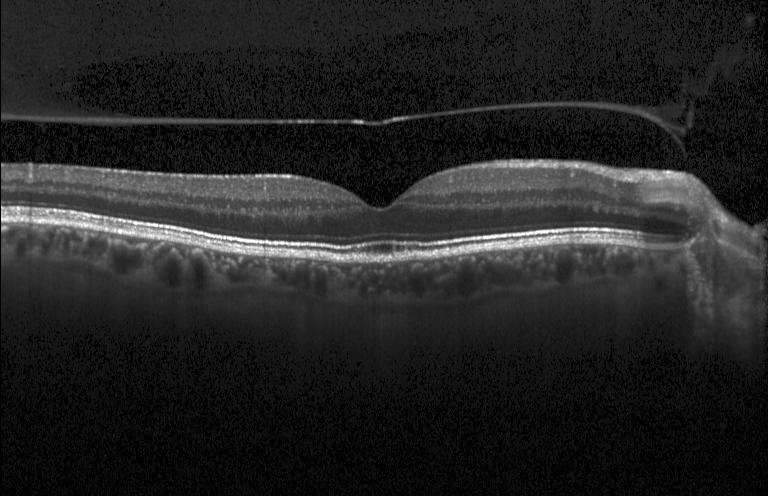
SD-OCT; macular scan; optical coherence tomography scan. Impression: no evidence of choroidal neovascularization, diabetic macular edema, or drusen.